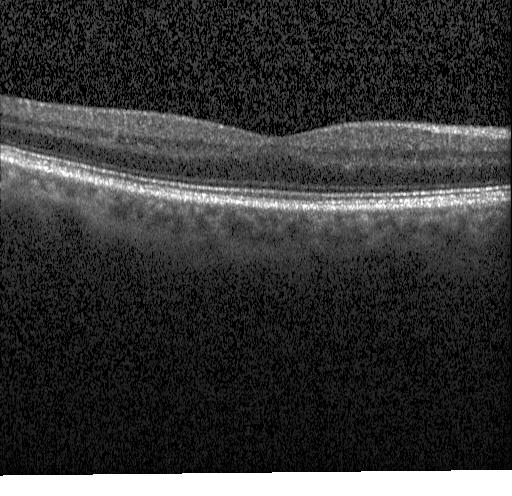 Spectral-domain OCT; retinal OCT B-scan. Dx: no choroidal neovascularization, diabetic macular edema, or drusen.